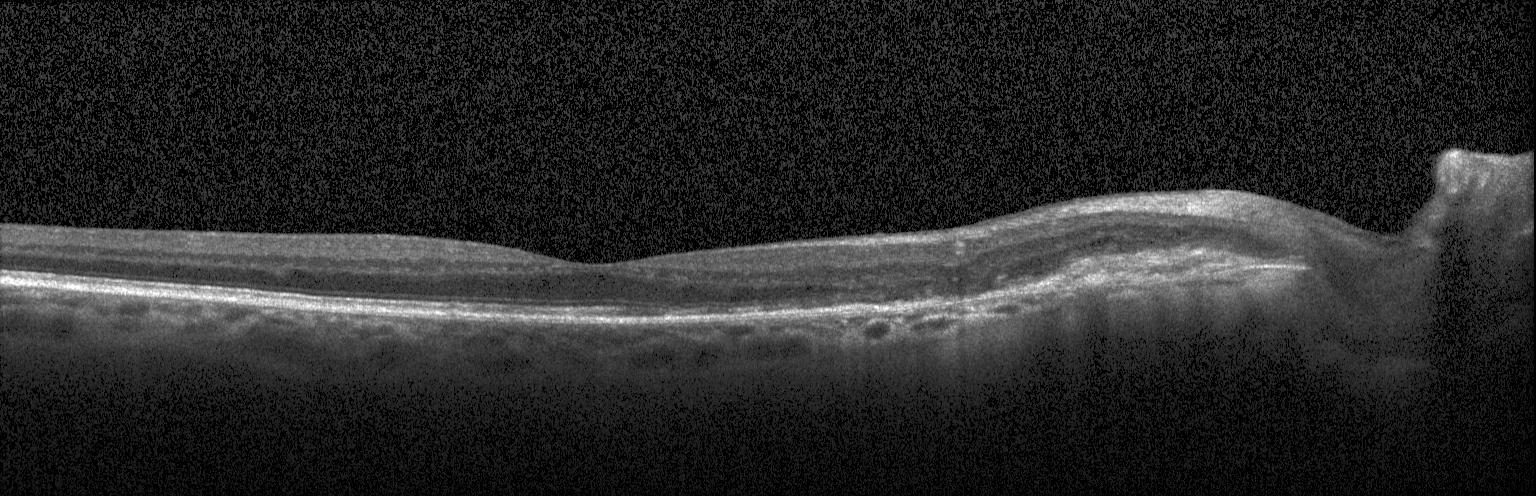

Optical coherence tomography scan — Diagnosis: a choroidal neovascular membrane.